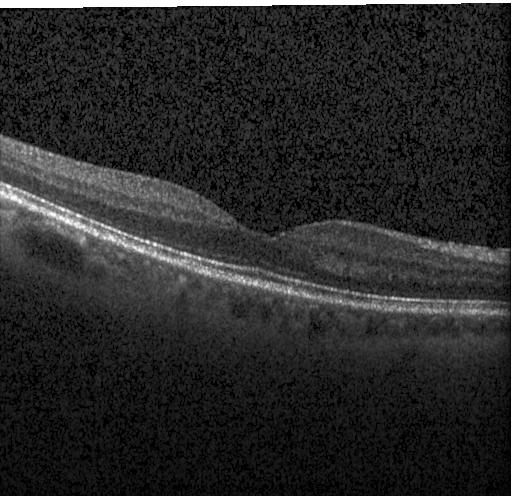

Assessment: neither choroidal neovascularization, diabetic macular edema, nor drusen.